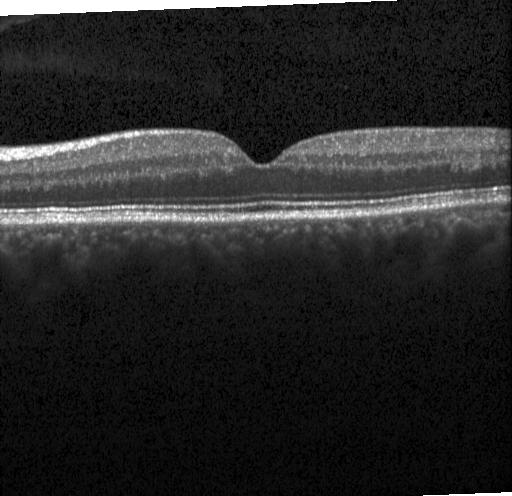
Retinal OCT B-scan — This B-scan demonstrates no evidence of CNV, DME, or drusen.